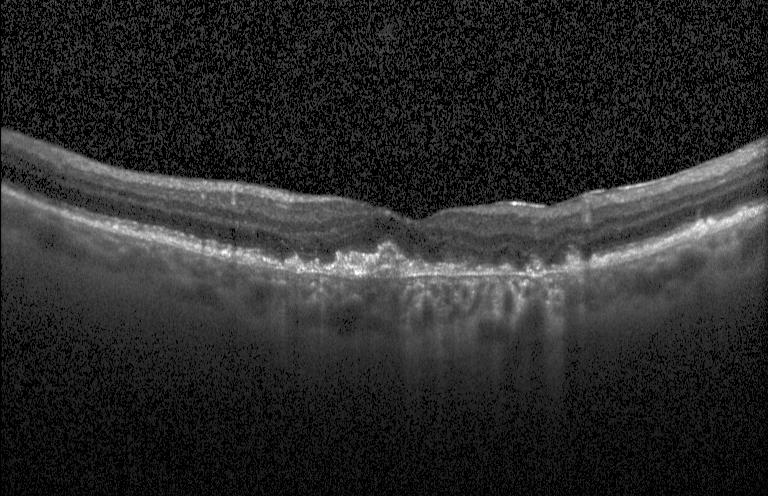
Heidelberg Spectralis; OCT B-scan; spectral-domain OCT; fovea-centered
Dx: a choroidal neovascular membrane.